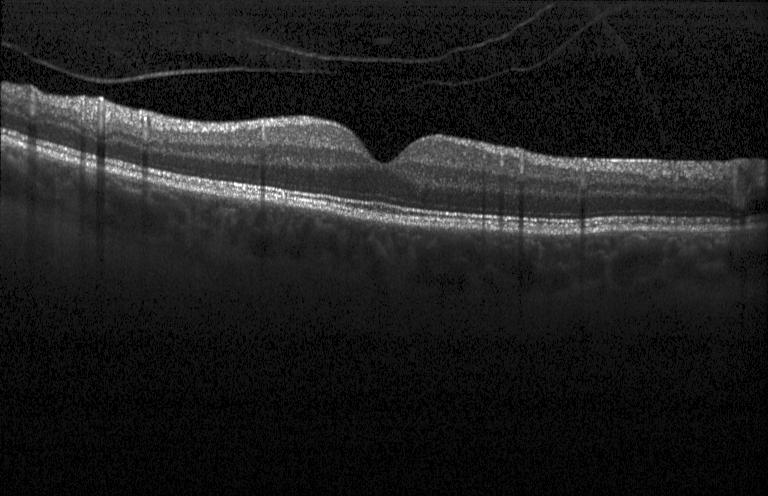
Macular scan, OCT B-scan. Impression: neither CNV, DME, nor drusen.